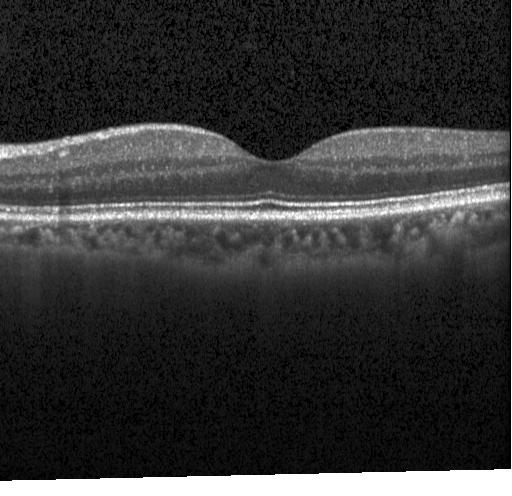 Spectral-domain optical coherence tomography, optical coherence tomography B-scan, centered on the fovea, instrument: Heidelberg Spectralis — Impression: no choroidal neovascularization, diabetic macular edema, or drusen.